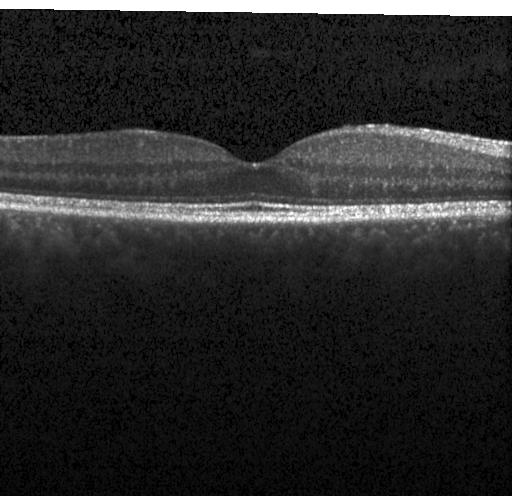 Finding: no evidence of choroidal neovascularization, diabetic macular edema, or drusen.